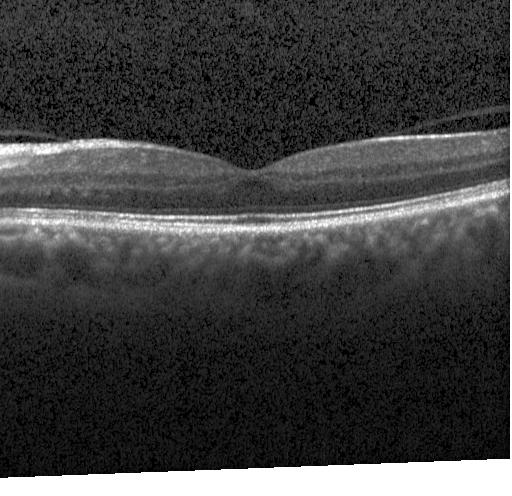 Macular scan · SD-OCT · OCT B-scan · Heidelberg Spectralis — No evidence of choroidal neovascularization, diabetic macular edema, or drusen.